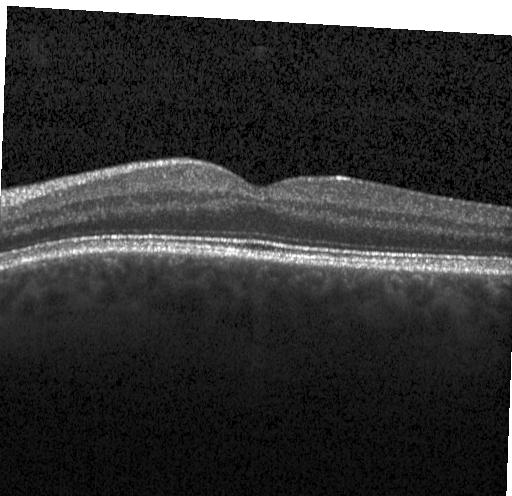
Acquired on a Heidelberg Spectralis · optical coherence tomography B-scan
OCT finding: no choroidal neovascularization, no diabetic macular edema, and no drusen.